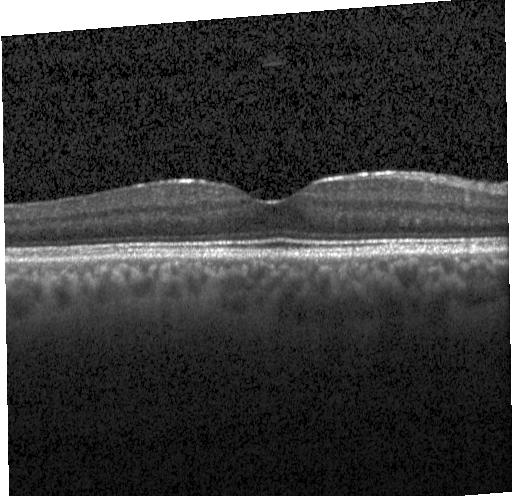
Retinal OCT B-scan; fovea-centered; SD-OCT; Heidelberg Spectralis OCT system.
Finding: no evidence of choroidal neovascularization, diabetic macular edema, or drusen.